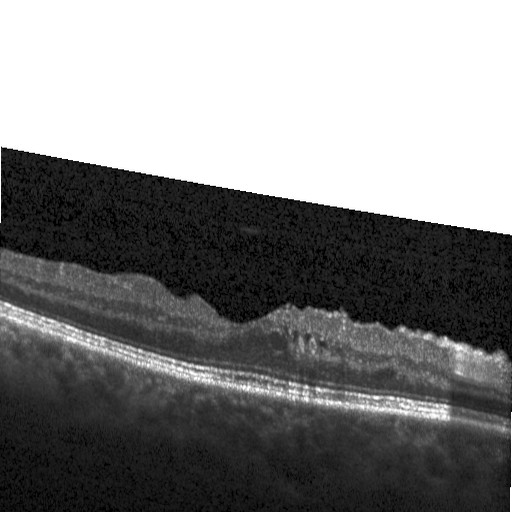

Optical coherence tomography B-scan · instrument: Heidelberg Spectralis · SD-OCT · horizontal scan through the fovea — DME.